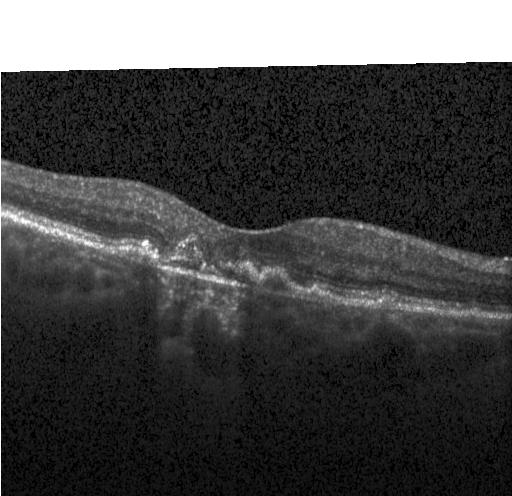
OCT line scan — Dx: a choroidal neovascular membrane.